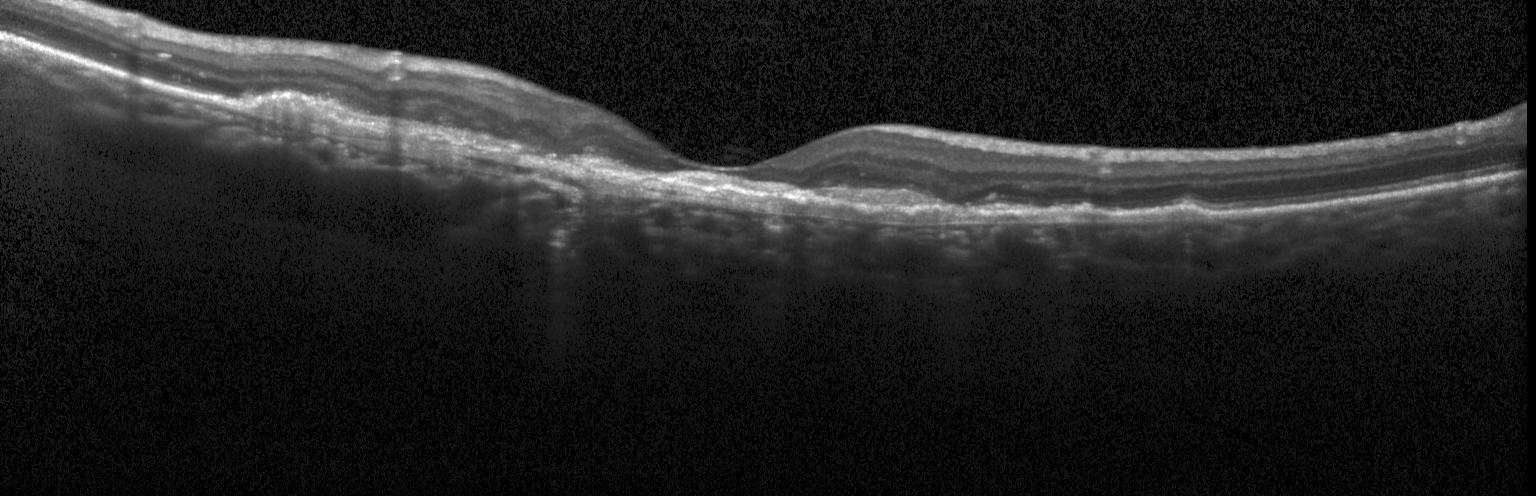 Macular scan. Retinal OCT cross-section.
OCT finding: choroidal neovascularization.